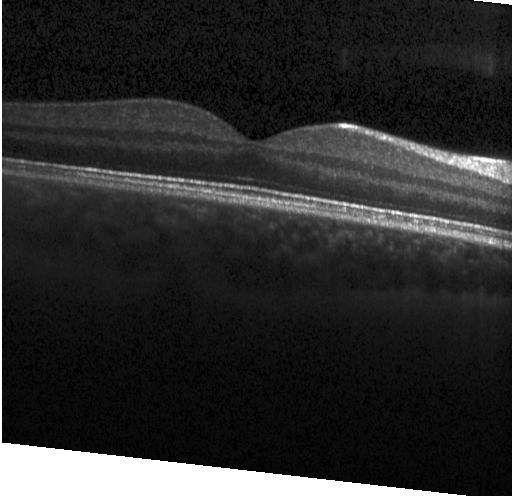

Finding: no evidence of choroidal neovascularization, diabetic macular edema, or drusen.